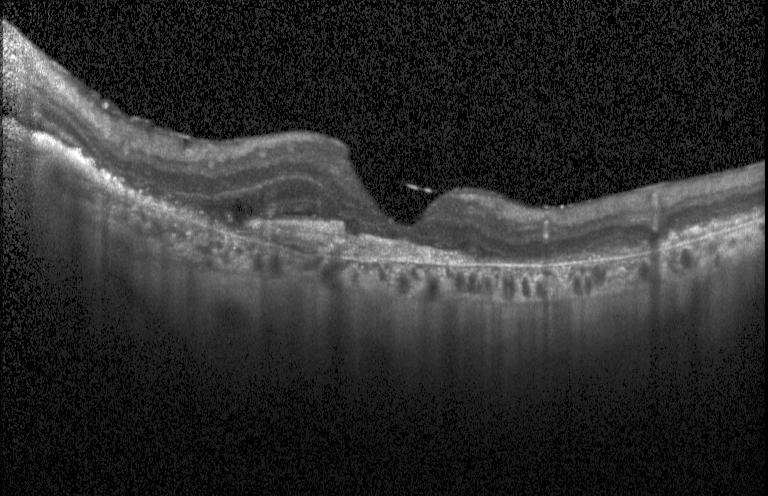
Finding: choroidal neovascularization.